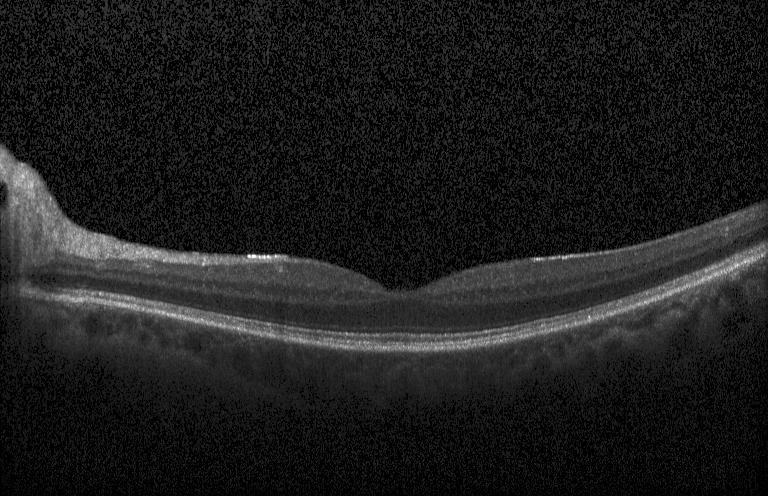
Spectral-domain OCT; optical coherence tomography B-scan. Impression: no choroidal neovascularization, no diabetic macular edema, and no drusen.